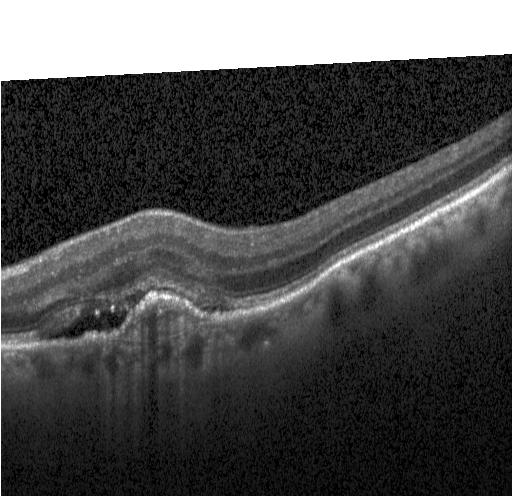 Centered on the fovea, Heidelberg Spectralis OCT system, retinal OCT B-scan.
Finding: a choroidal neovascular membrane.